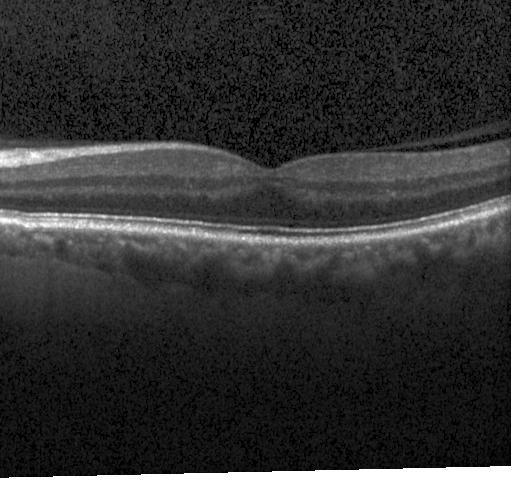
OCT B-scan; Heidelberg Spectralis.
Impression: no evidence of CNV, DME, or drusen.